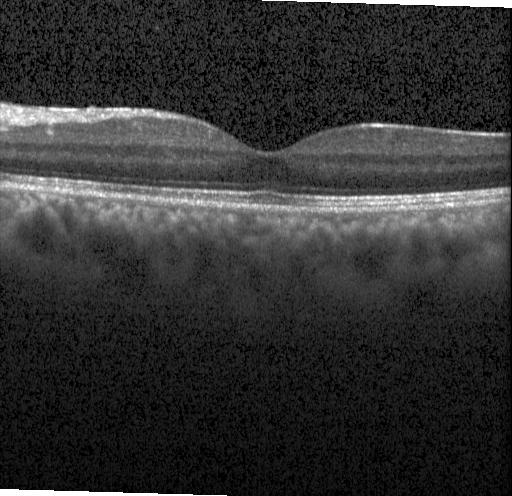
Spectral-domain optical coherence tomography. Retinal OCT cross-section — Finding: no choroidal neovascularization, no diabetic macular edema, and no drusen.